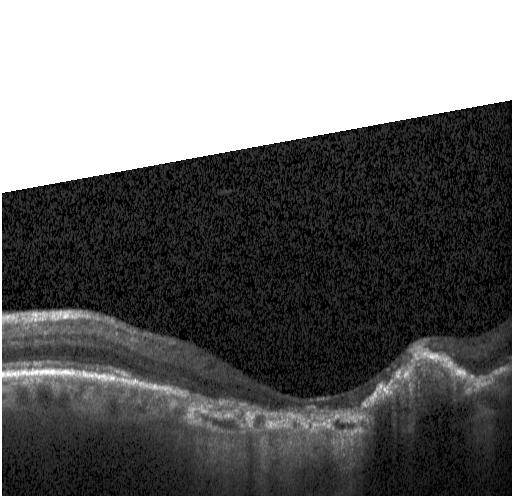

Assessment: a choroidal neovascular membrane.